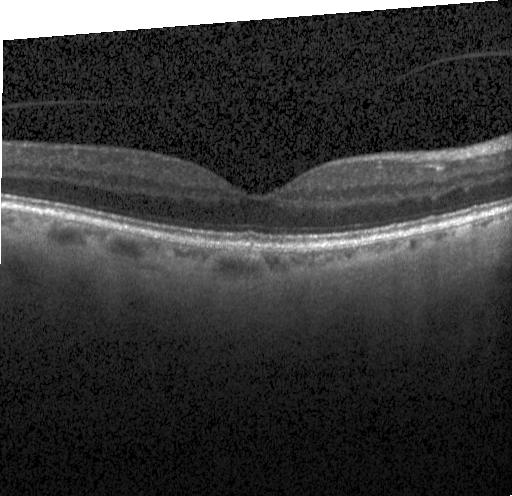 Retinal OCT B-scan
Finding: no evidence of choroidal neovascularization, diabetic macular edema, or drusen.